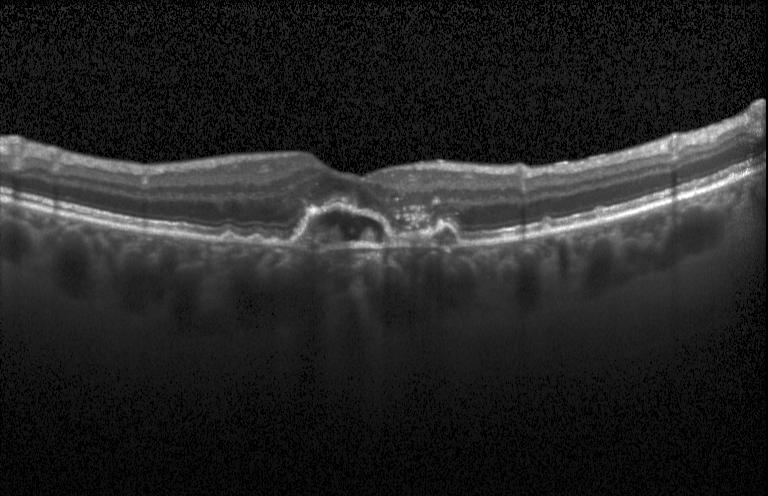 Retinal OCT cross-section showing a choroidal neovascular membrane.